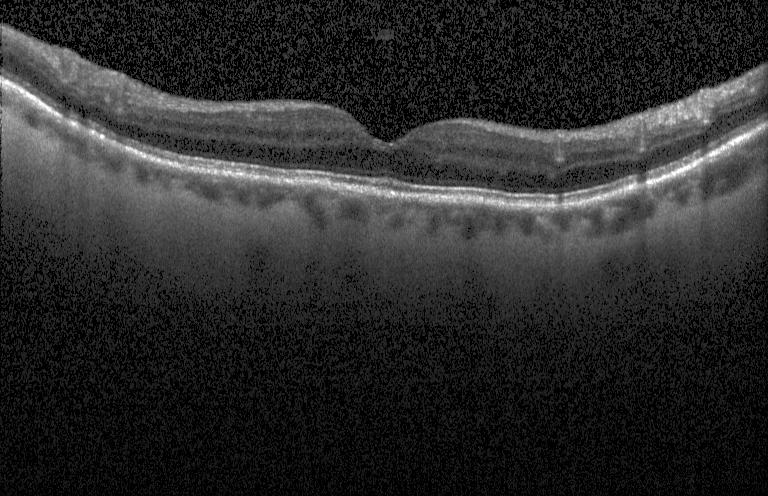
Instrument: Heidelberg Spectralis · spectral-domain OCT · retinal OCT B-scan. The scan shows no CNV, DME, or drusen.